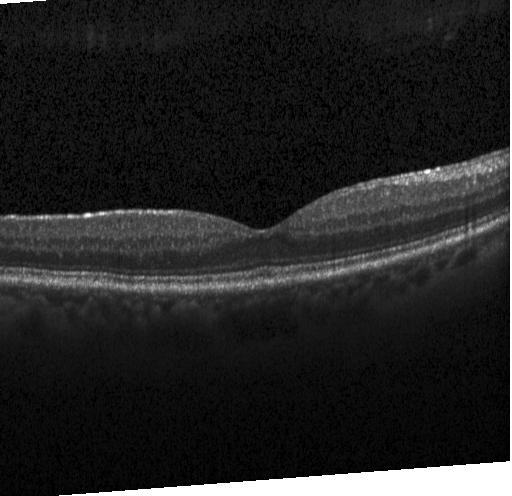 Retinal OCT cross-section; instrument: Heidelberg Spectralis.
Finding: no CNV, no DME, and no drusen.